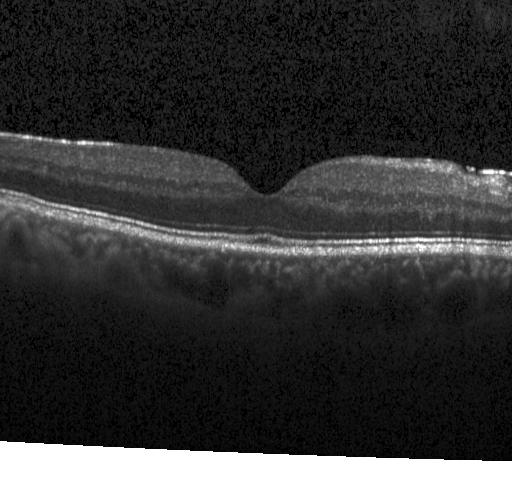

Macular scan. Retinal OCT B-scan. Macular OCT: no evidence of choroidal neovascularization, diabetic macular edema, or drusen.